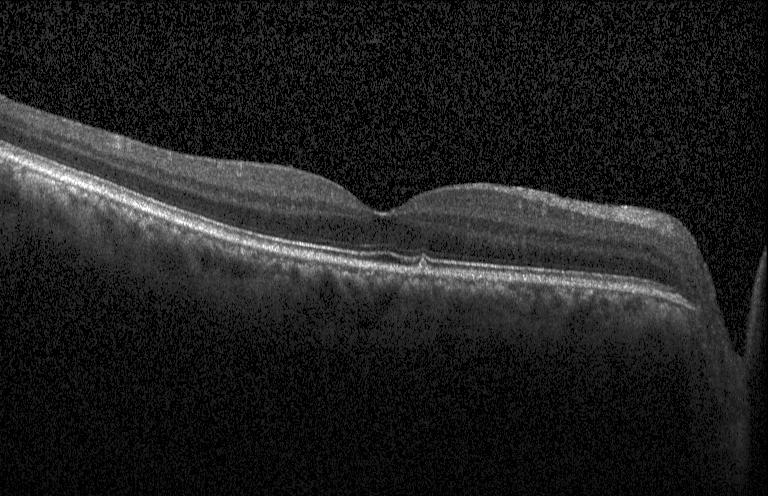
Acquired on a Heidelberg Spectralis, retinal OCT cross-section
Finding: sub-RPE drusenoid deposits.